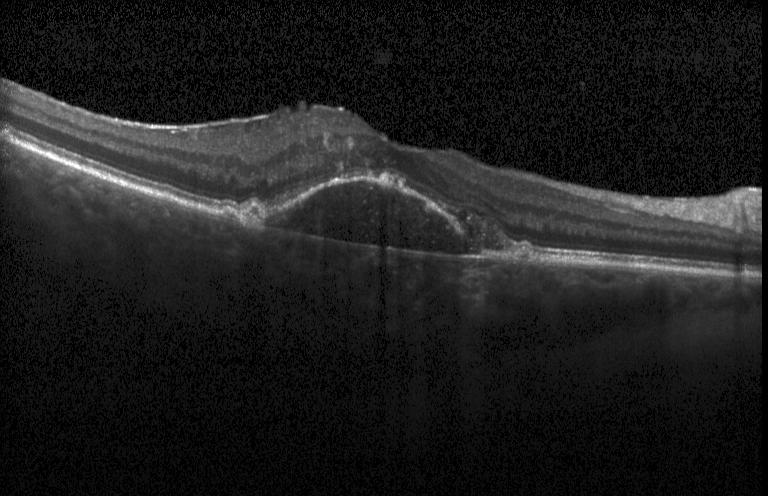 SD-OCT · OCT B-scan · centered on the fovea · acquired on a Heidelberg Spectralis.
Diagnosis: choroidal neovascularization (CNV).